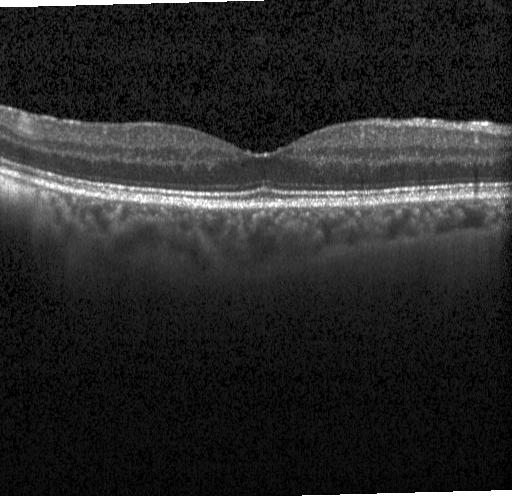

Retinal OCT cross-section. Macular scan. SD-OCT. Heidelberg Spectralis.
Neither choroidal neovascularization, diabetic macular edema, nor drusen.